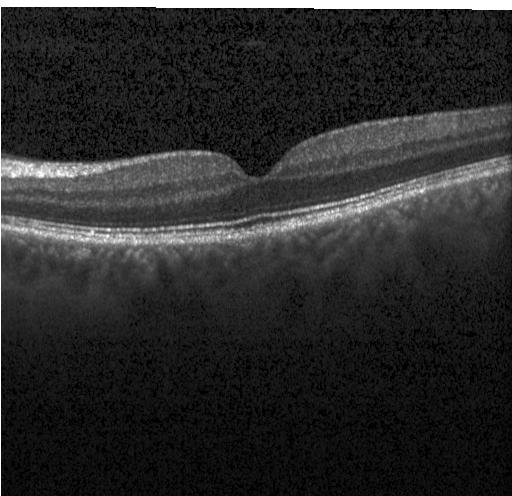 OCT line scan.
The scan shows no choroidal neovascularization, diabetic macular edema, or drusen.